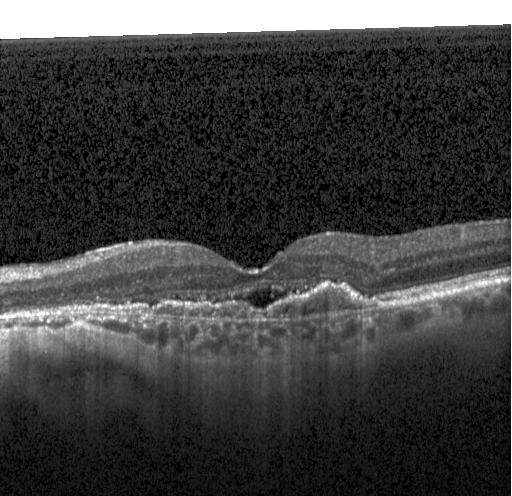

Diagnosis: choroidal neovascularization (CNV).